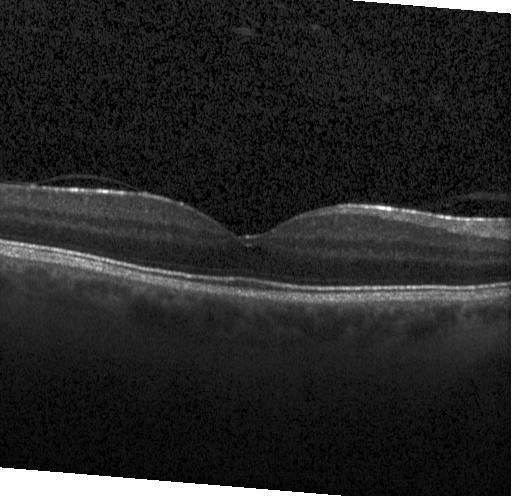

Optical coherence tomography B-scan. Spectral-domain optical coherence tomography. Through the macula — Macular OCT: no evidence of choroidal neovascularization, diabetic macular edema, or drusen.